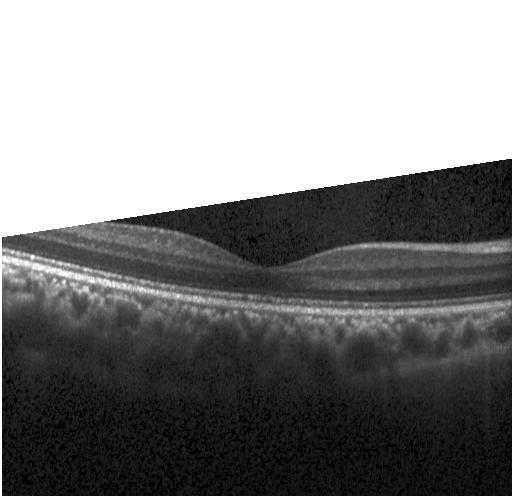 Acquired on a Heidelberg Spectralis; centered on the fovea; retinal OCT B-scan; SD-OCT. Finding: no choroidal neovascularization, diabetic macular edema, or drusen.